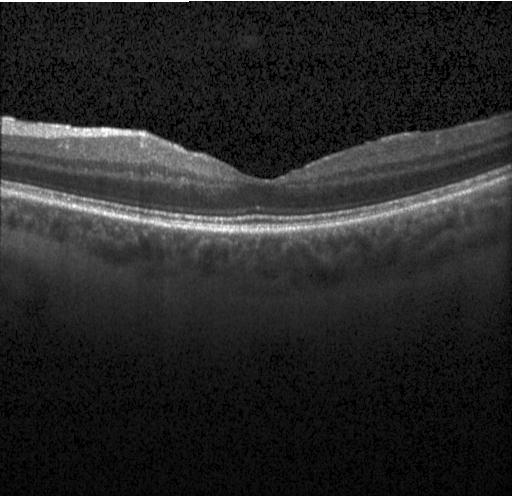

This B-scan demonstrates no choroidal neovascularization, diabetic macular edema, or drusen.